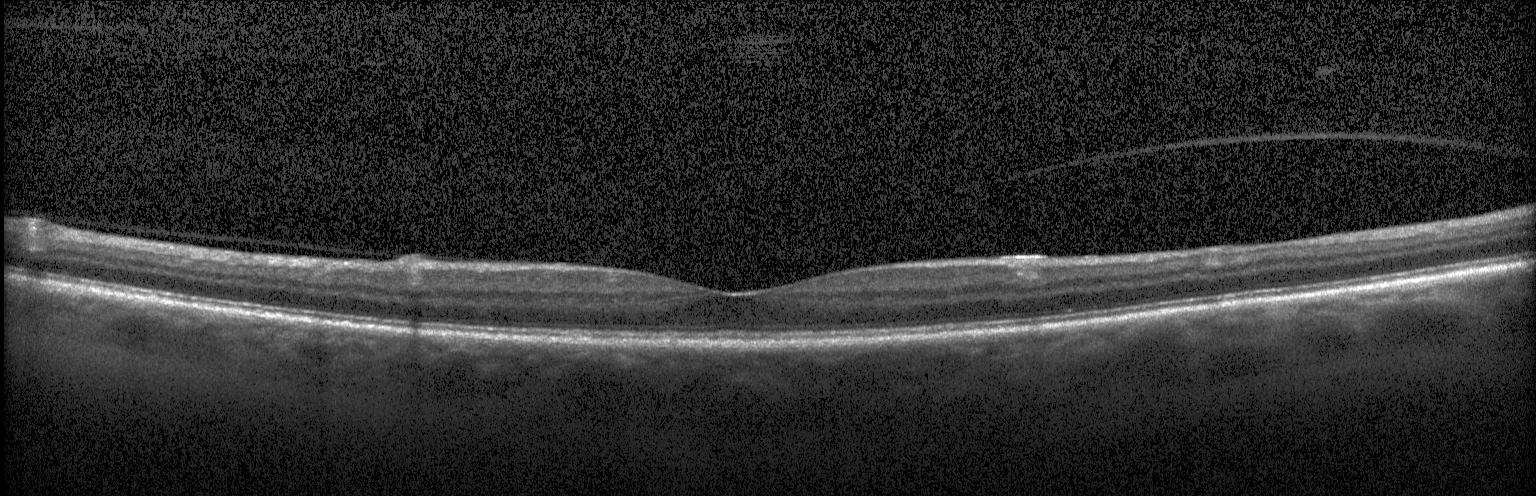
Retinal OCT B-scan, instrument: Heidelberg Spectralis, horizontal scan through the fovea
Macular OCT: no CNV, DME, or drusen.